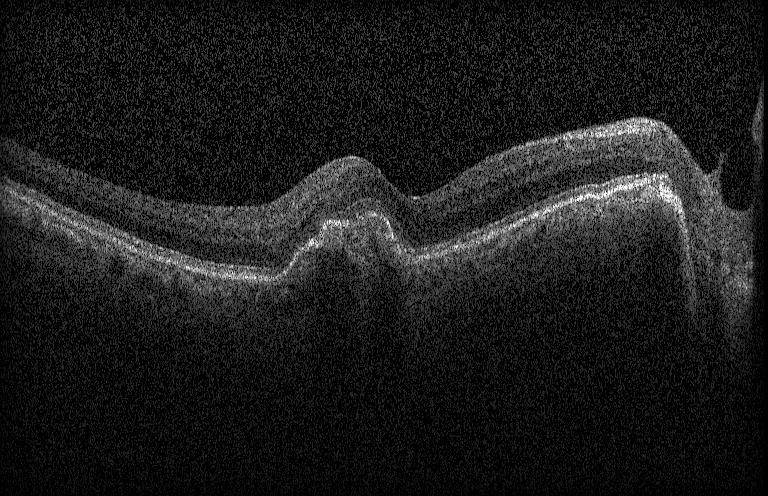
OCT line scan. Horizontal scan through the fovea — This B-scan demonstrates choroidal neovascularization.